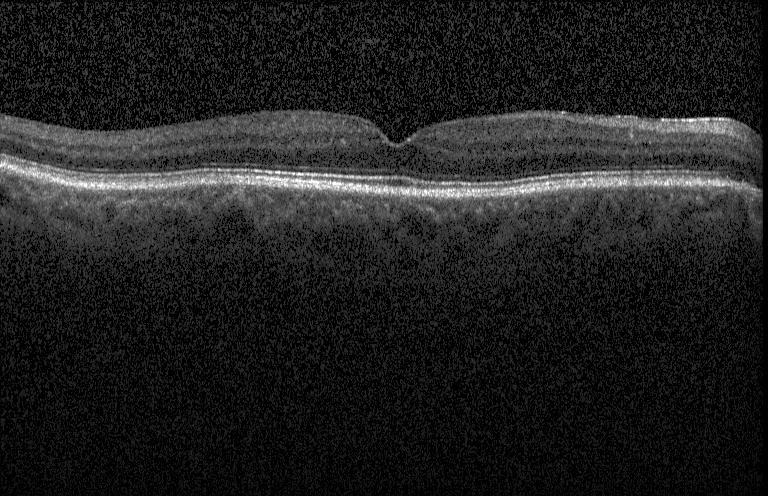 Optical coherence tomography scan, Heidelberg Spectralis, horizontal scan through the fovea. Impression: no evidence of choroidal neovascularization, diabetic macular edema, or drusen.